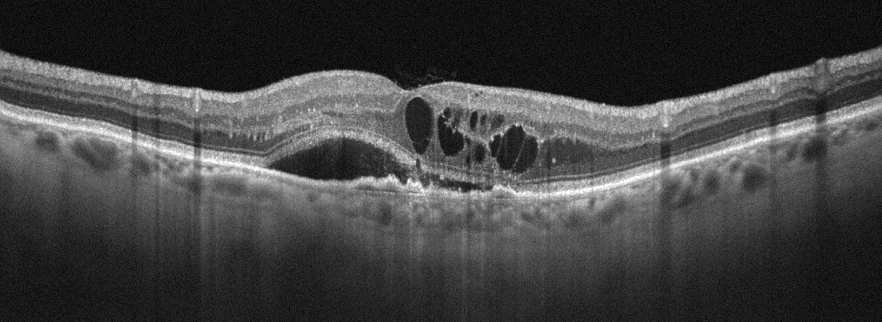 OCT B-scan. Optovue Avanti RTVue XR. Fovea-centered. Left eye
Finding: age-related macular degeneration.